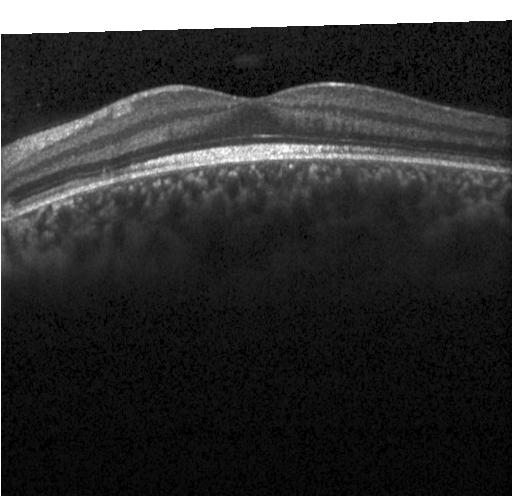
Horizontal scan through the fovea. OCT line scan. SD-OCT. Instrument: Heidelberg Spectralis
Finding: neither CNV, DME, nor drusen.